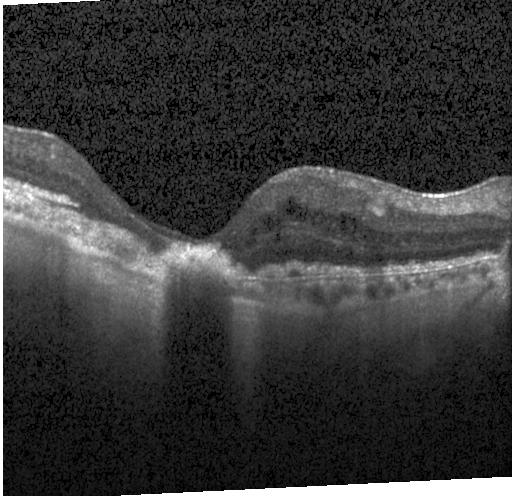
OCT line scan; instrument: Heidelberg Spectralis; spectral-domain optical coherence tomography. This B-scan demonstrates choroidal neovascularization (CNV).